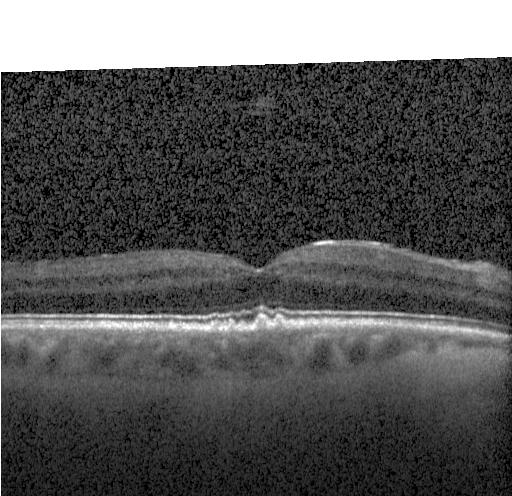 Optical coherence tomography scan. Heidelberg Spectralis. Horizontal scan through the fovea. Impression: sub-RPE drusenoid deposits.